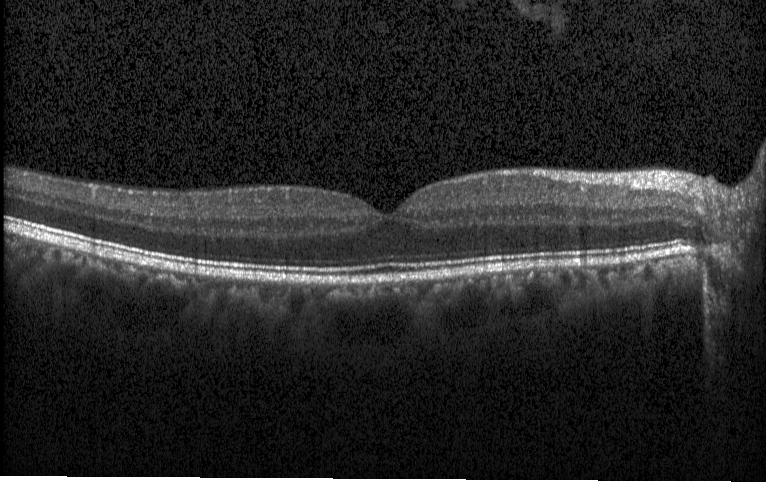 OCT B-scan showing no choroidal neovascularization, diabetic macular edema, or drusen.